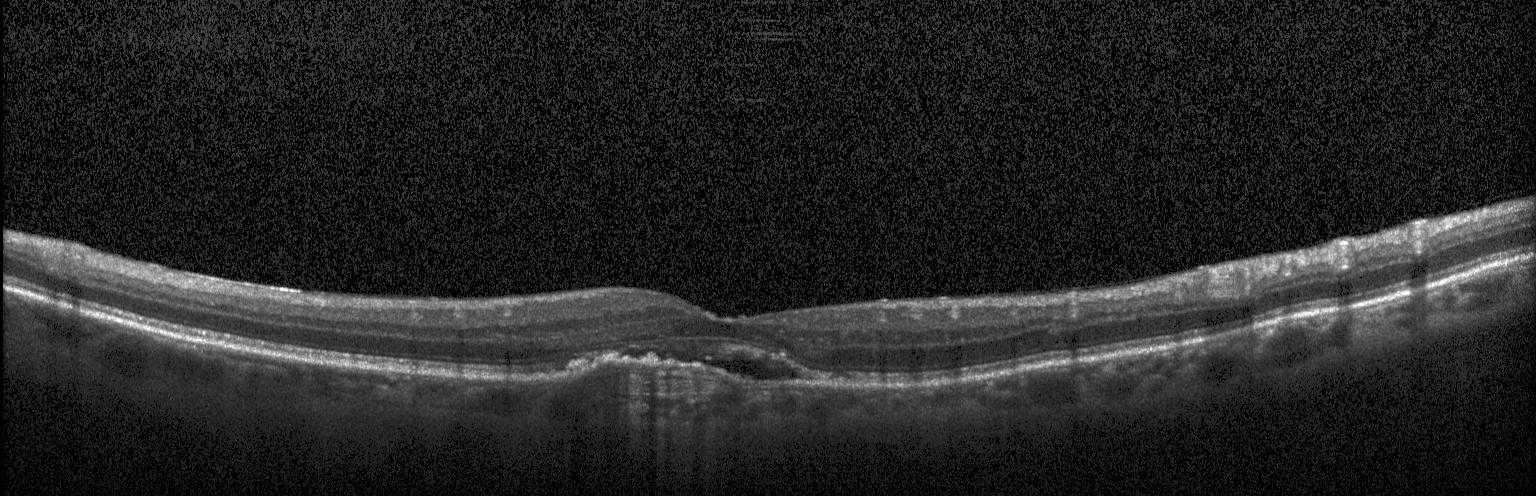
Retinal OCT B-scan. Impression: a choroidal neovascular membrane.